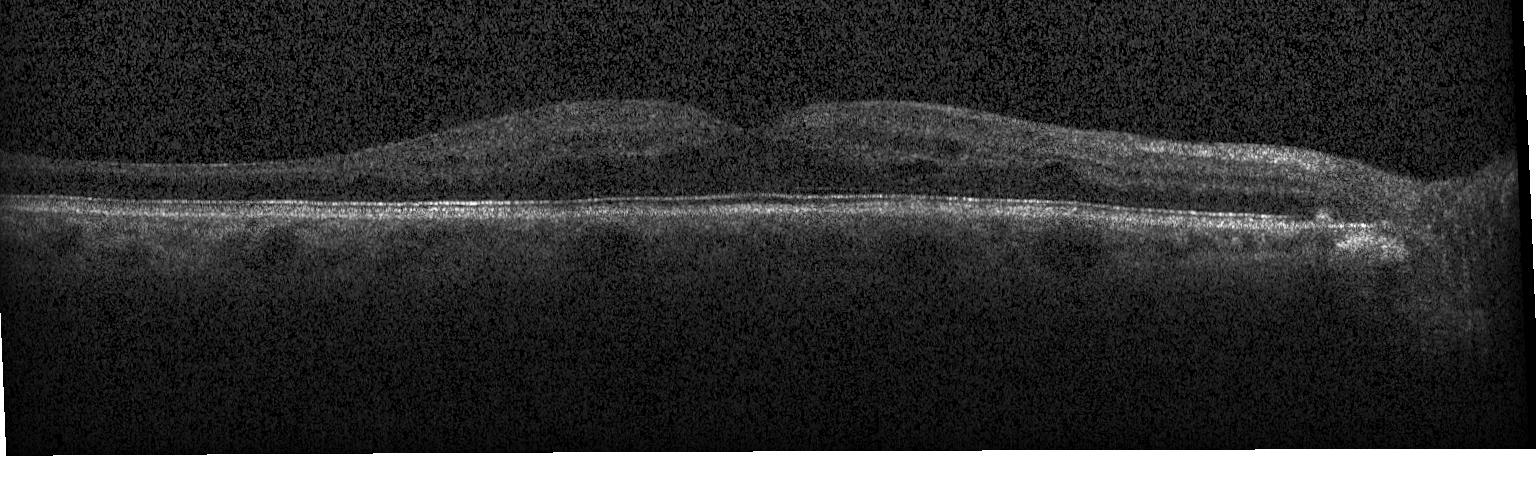 OCT line scan · spectral-domain OCT · through the macula · Heidelberg Spectralis. Diagnosis: DME.